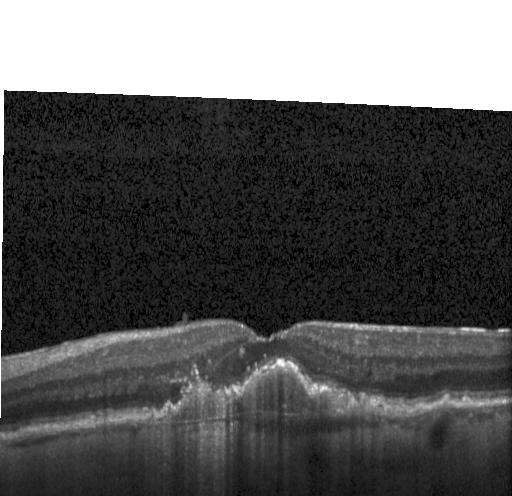 Spectral-domain OCT B-scan: choroidal neovascularization.